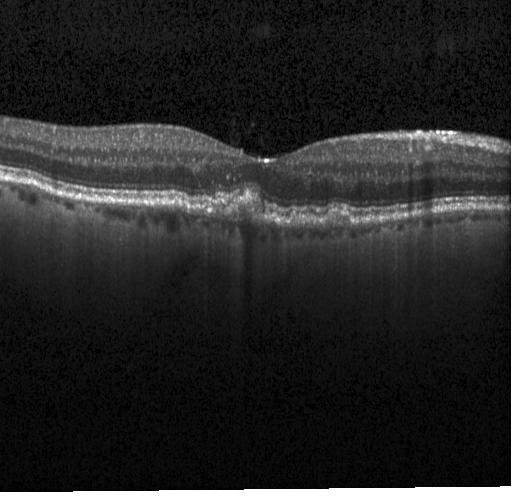 Acquired on a Heidelberg Spectralis, macular scan, optical coherence tomography B-scan, spectral-domain OCT. OCT finding: multiple drusen.